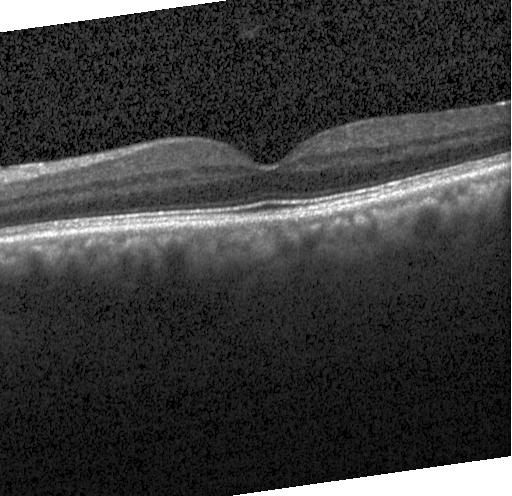

OCT B-scan; centered on the fovea — Finding: no choroidal neovascularization, diabetic macular edema, or drusen.